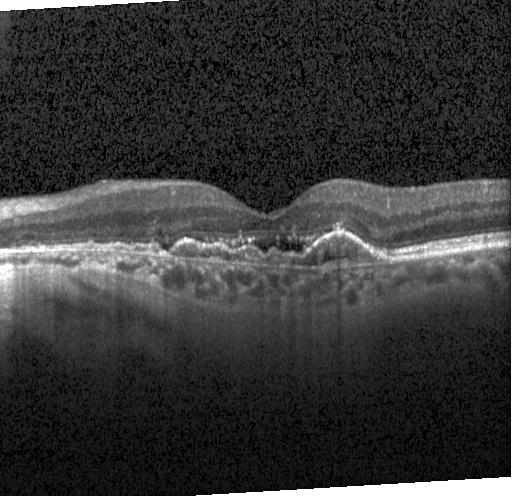 Retinal OCT B-scan, instrument: Heidelberg Spectralis
Diagnosis: a choroidal neovascular membrane.